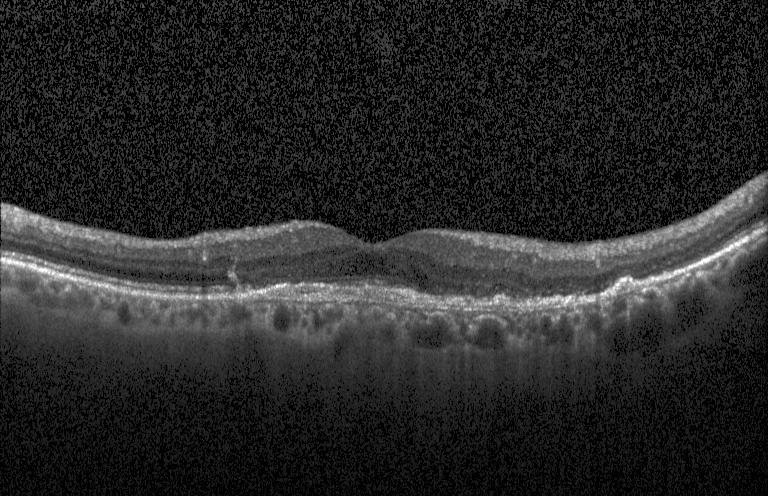
Retinal OCT B-scan · through the macula
Macular OCT: CNV.